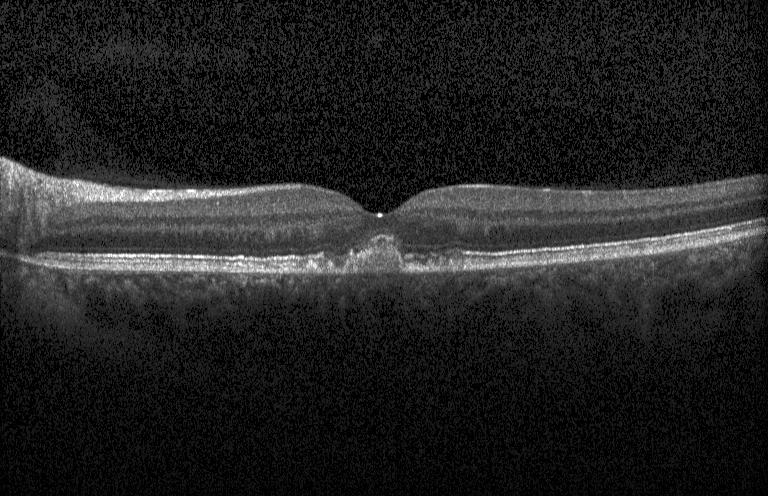 OCT line scan; fovea-centered; spectral-domain OCT; Heidelberg Spectralis OCT system — Finding: sub-RPE drusenoid deposits.